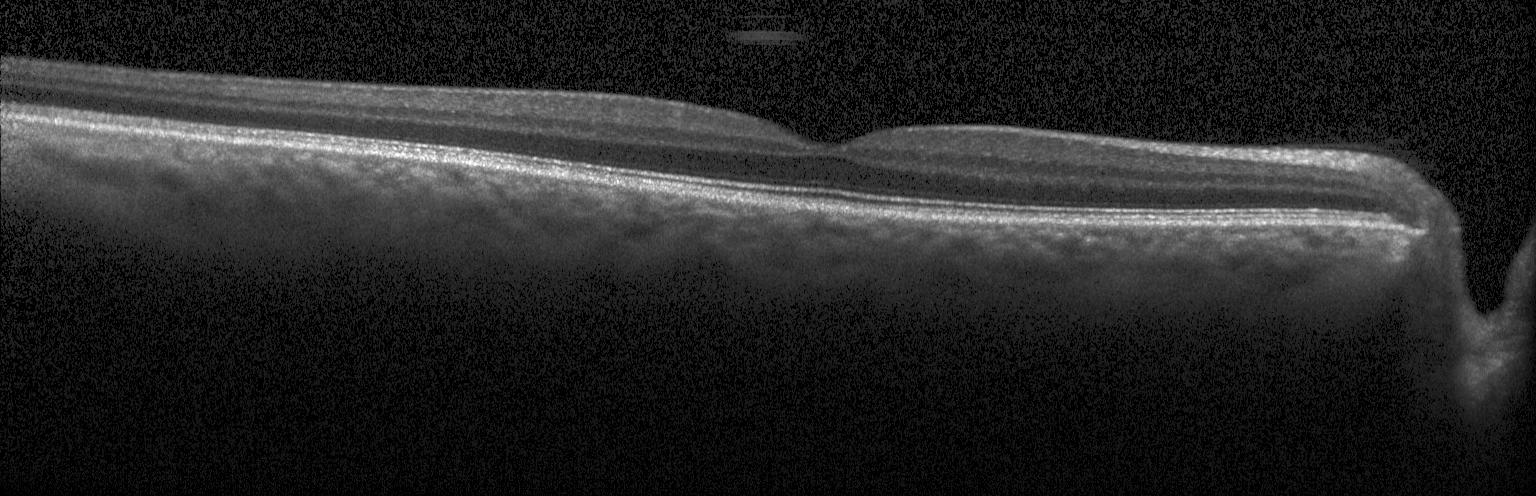

OCT B-scan, horizontal scan through the fovea, SD-OCT — Impression: no evidence of choroidal neovascularization, diabetic macular edema, or drusen.